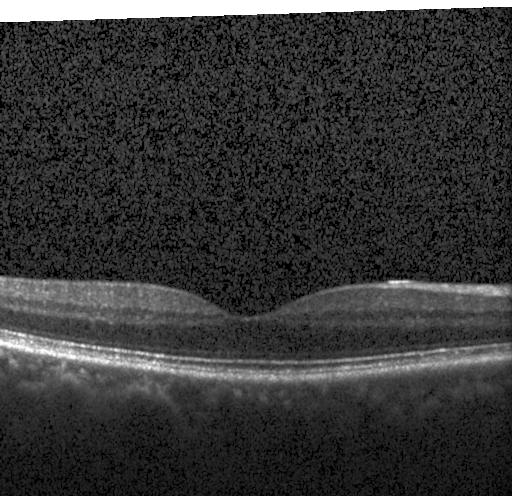 Impression: neither choroidal neovascularization, diabetic macular edema, nor drusen.